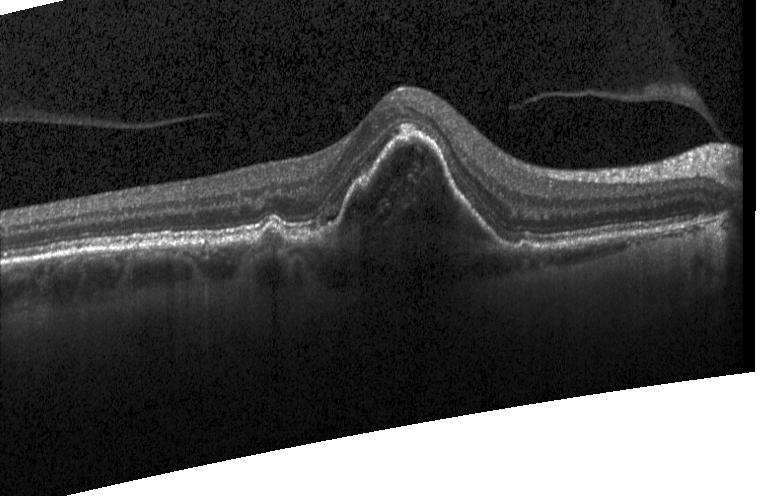
Finding: a choroidal neovascular membrane.